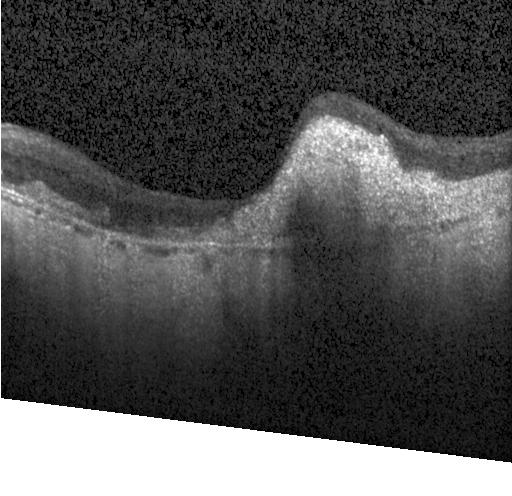
Finding: choroidal neovascularization (CNV).